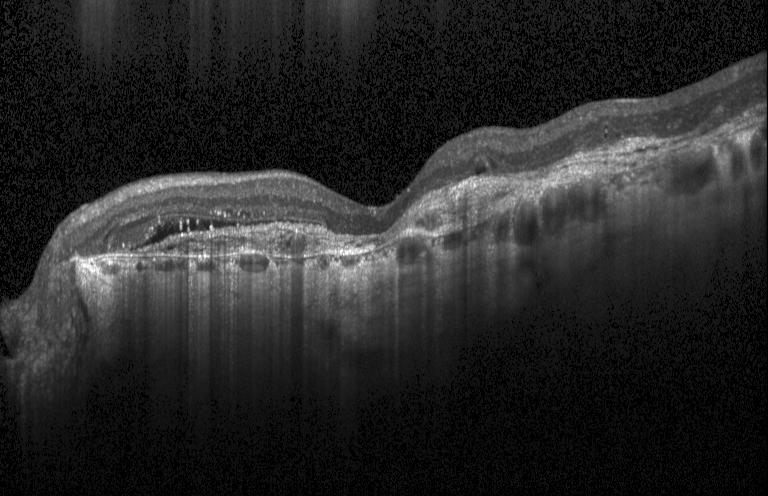 Spectral-domain OCT. Optical coherence tomography B-scan. Fovea-centered
Diagnosis: a choroidal neovascular membrane.